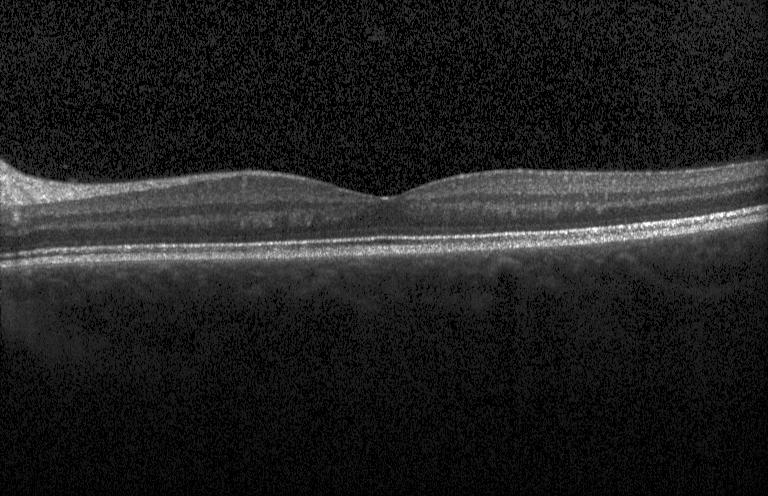 Retinal OCT cross-section; spectral-domain optical coherence tomography — Impression: no choroidal neovascularization, no diabetic macular edema, and no drusen.